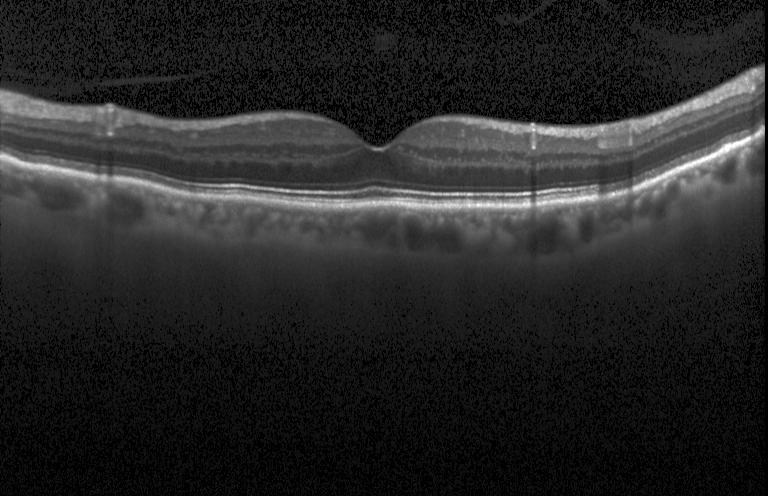 Macular OCT: no evidence of choroidal neovascularization, diabetic macular edema, or drusen.